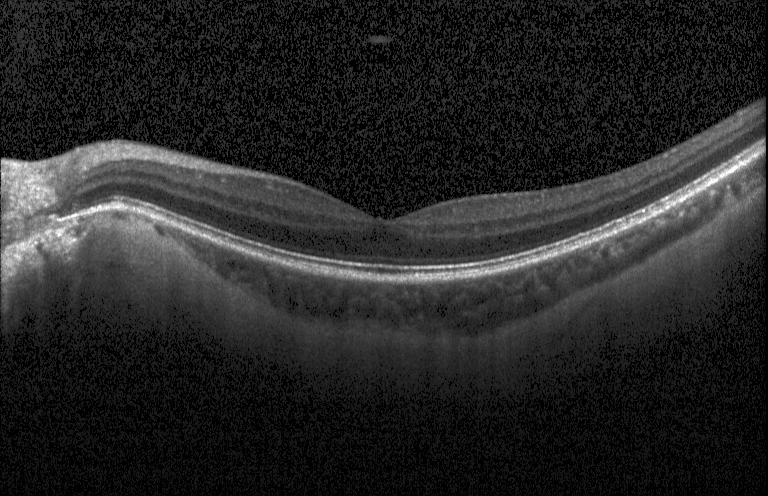 Heidelberg Spectralis OCT system; horizontal scan through the fovea; retinal OCT cross-section
Diagnosis: no choroidal neovascularization, no diabetic macular edema, and no drusen.